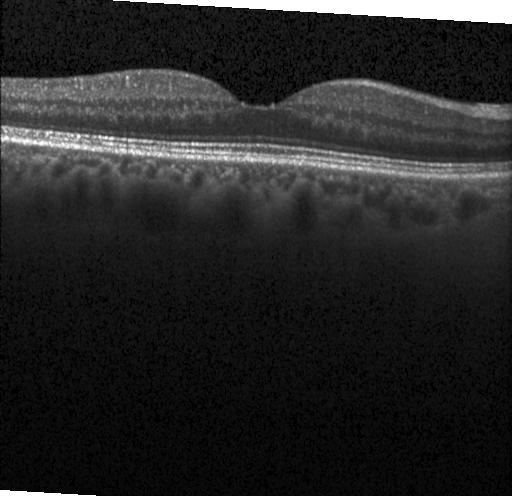

Retinal OCT B-scan.
The scan shows no evidence of CNV, DME, or drusen.